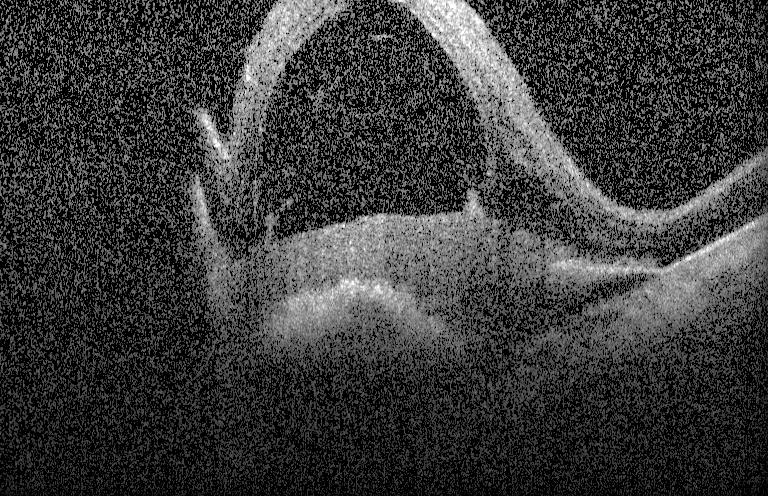 Spectral-domain OCT B-scan: CNV.